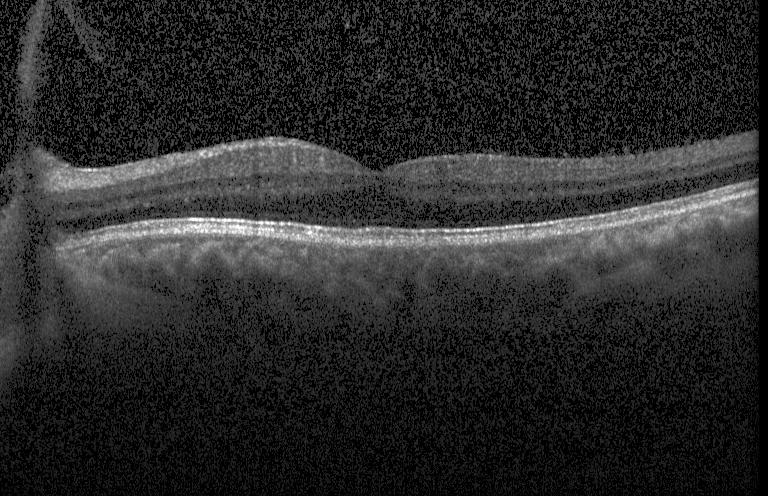
Retinal OCT cross-section, spectral-domain optical coherence tomography, Heidelberg Spectralis OCT system, through the macula
Finding: no choroidal neovascularization, diabetic macular edema, or drusen.